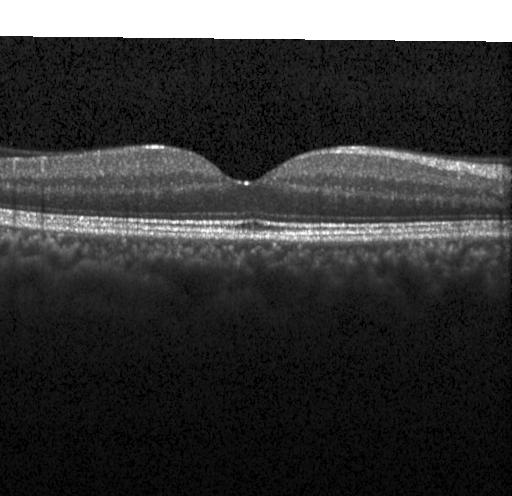
Optical coherence tomography scan. The scan shows no choroidal neovascularization, no diabetic macular edema, and no drusen.